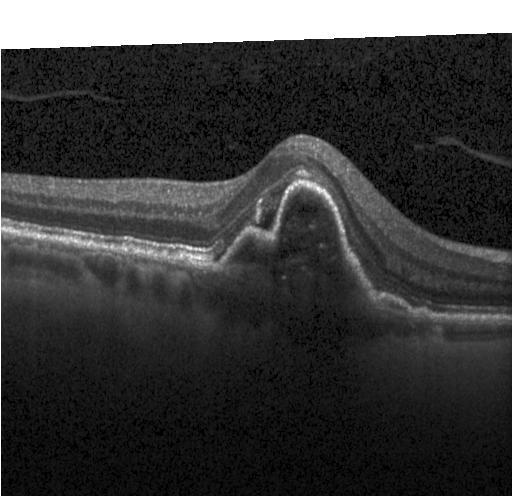

Diagnosis: a choroidal neovascular membrane.